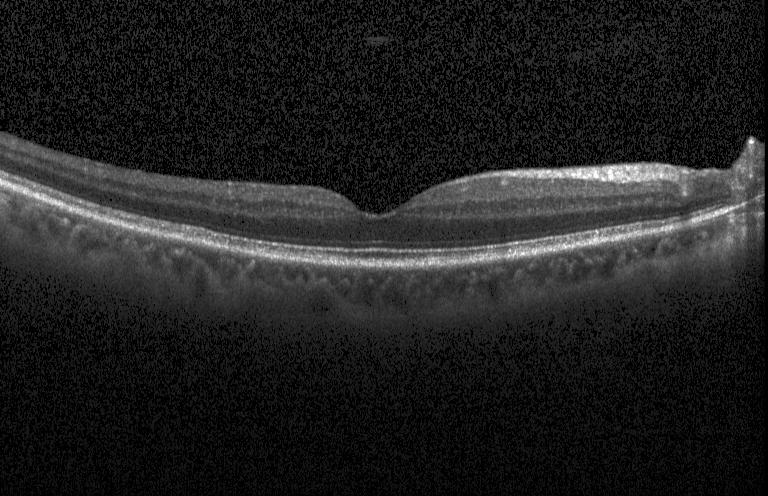 Acquired on a Heidelberg Spectralis · optical coherence tomography B-scan · spectral-domain OCT · through the macula. Finding: no evidence of choroidal neovascularization, diabetic macular edema, or drusen.